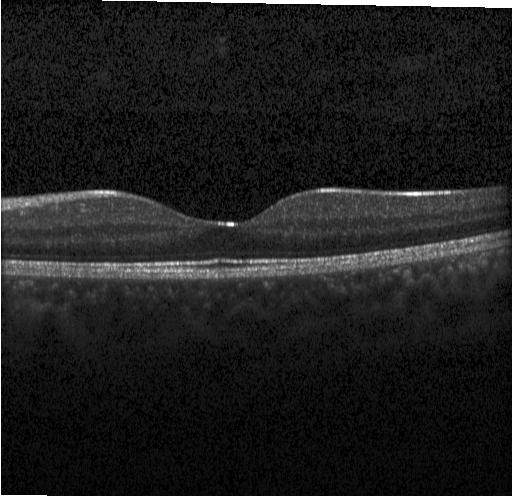
Optical coherence tomography scan, acquired on a Heidelberg Spectralis, spectral-domain OCT.
Diagnosis: no evidence of choroidal neovascularization, diabetic macular edema, or drusen.